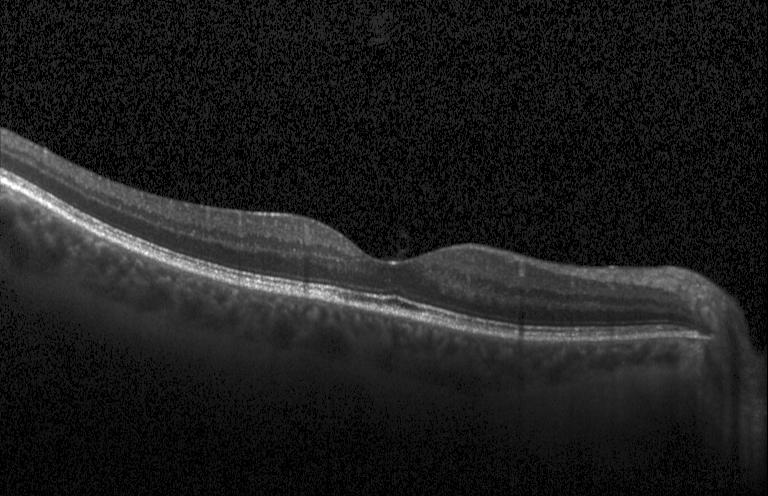

Optical coherence tomography B-scan. Acquired on a Heidelberg Spectralis.
OCT finding: no choroidal neovascularization, no diabetic macular edema, and no drusen.